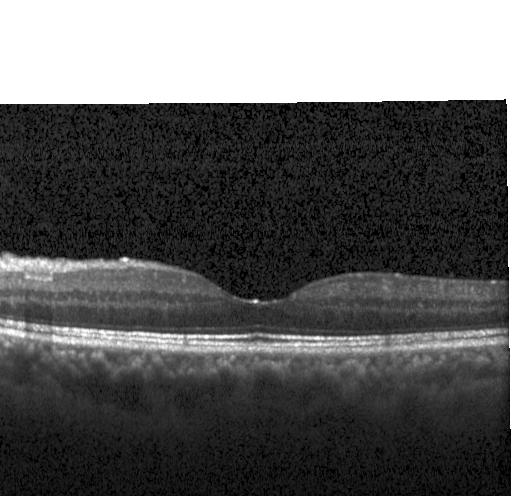
Retinal OCT B-scan. Spectral-domain OCT. Through the macula. Impression: no choroidal neovascularization, no diabetic macular edema, and no drusen.